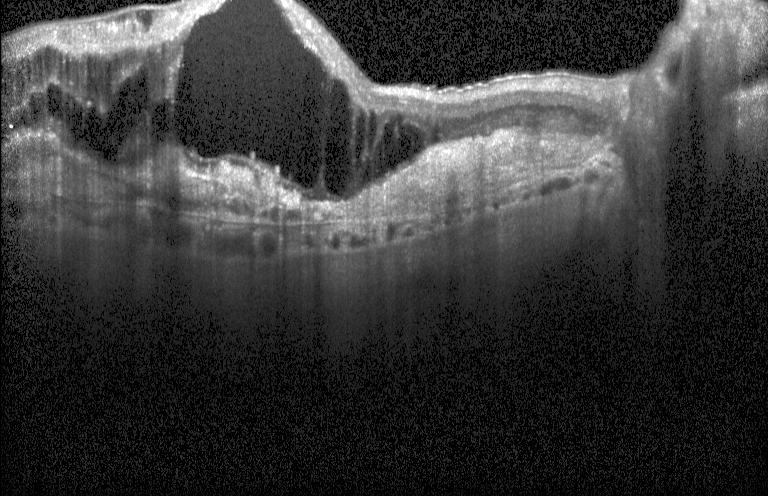 This B-scan demonstrates choroidal neovascularization.